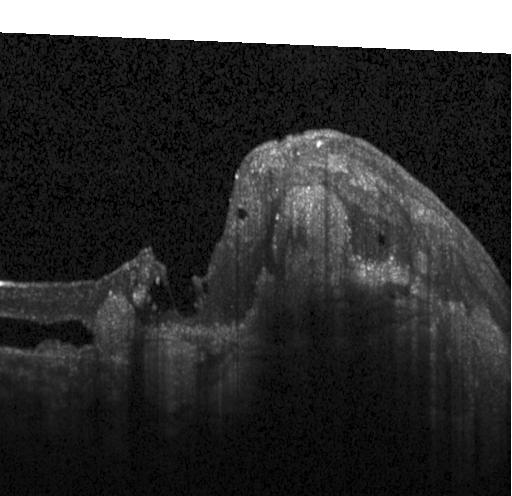 Choroidal neovascularization.